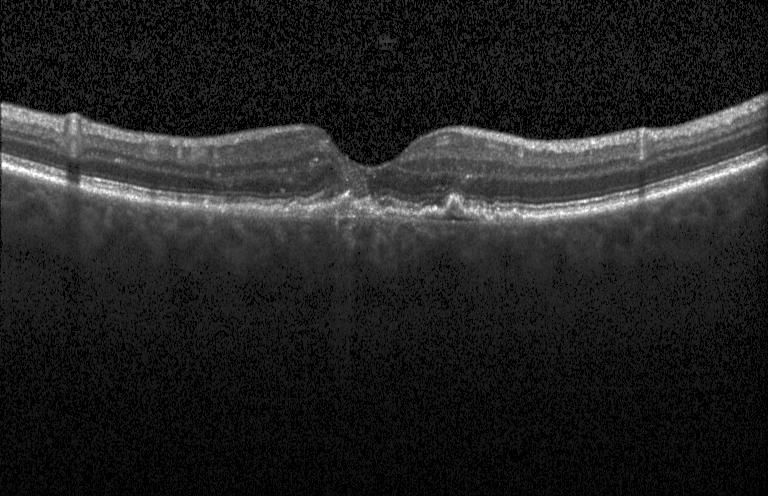 Instrument: Heidelberg Spectralis, horizontal scan through the fovea, optical coherence tomography B-scan — Dx: choroidal neovascularization (CNV).